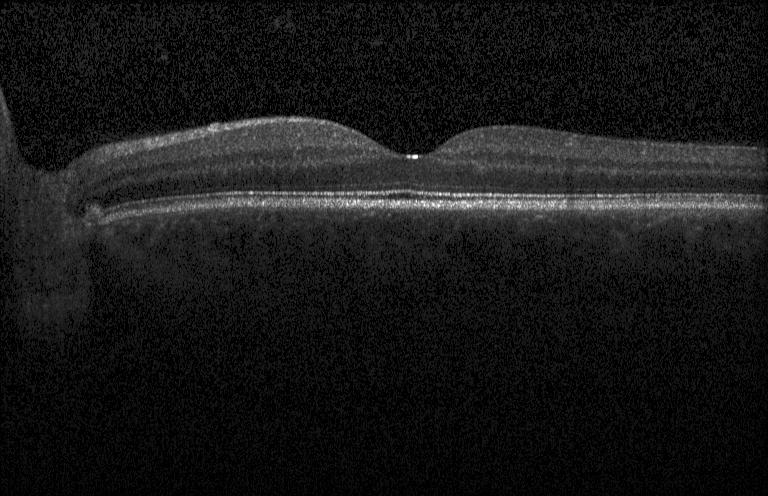 Retinal OCT cross-section
The scan shows neither choroidal neovascularization, diabetic macular edema, nor drusen.